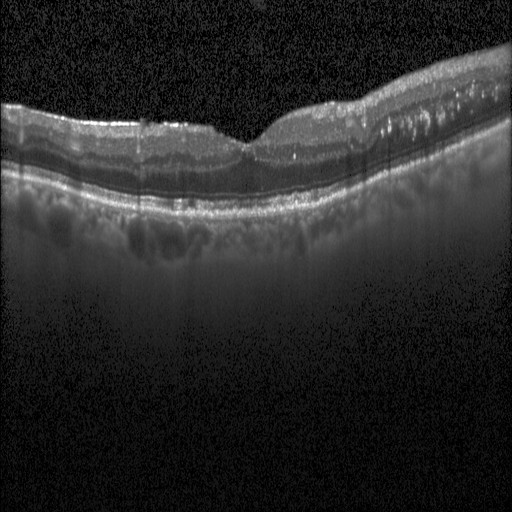

Spectral-domain OCT B-scan: diabetic macular edema (DME).